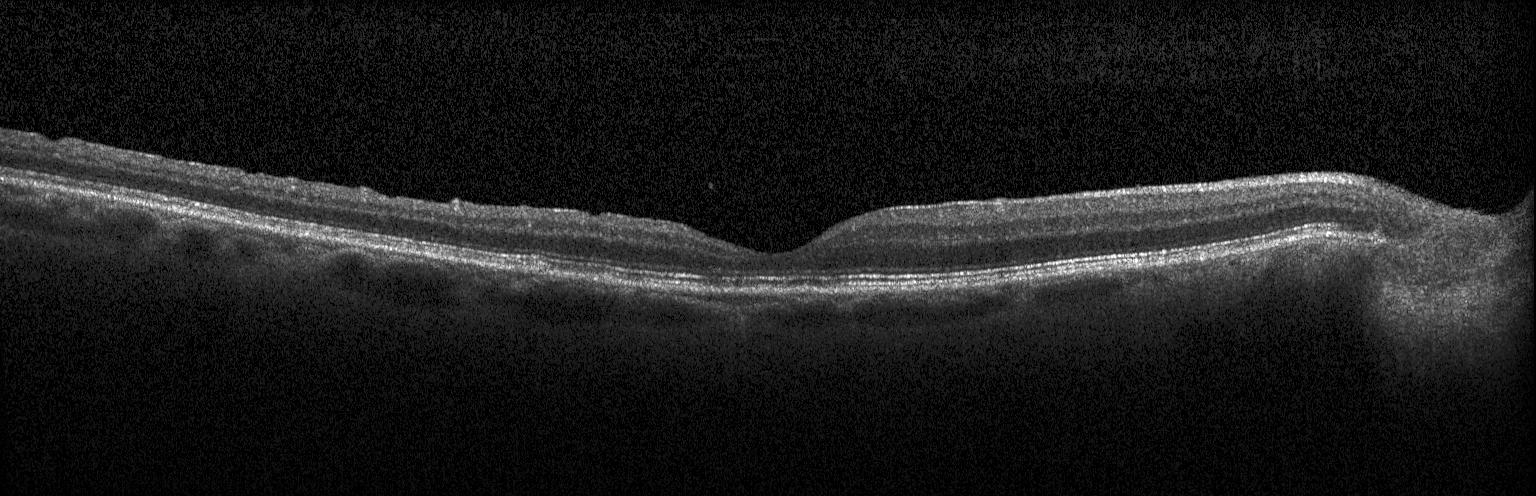
This B-scan demonstrates no evidence of choroidal neovascularization, diabetic macular edema, or drusen.